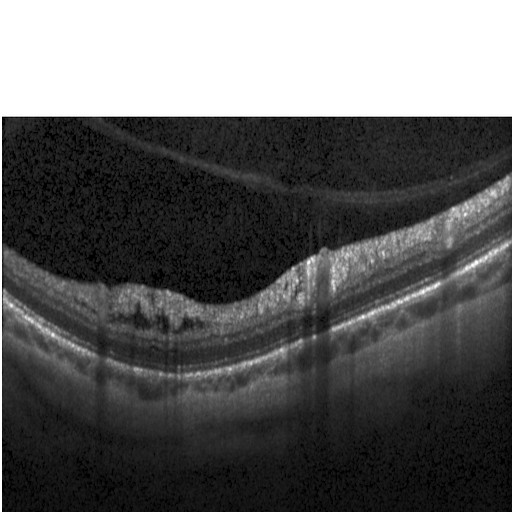

Heidelberg Spectralis · horizontal scan through the fovea · OCT B-scan · SD-OCT.
Finding: diabetic macular edema.